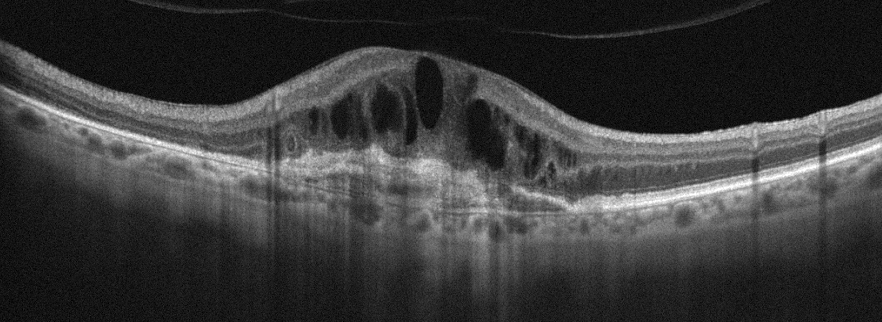 OD. Optical coherence tomography scan.
OCT finding: AMD.